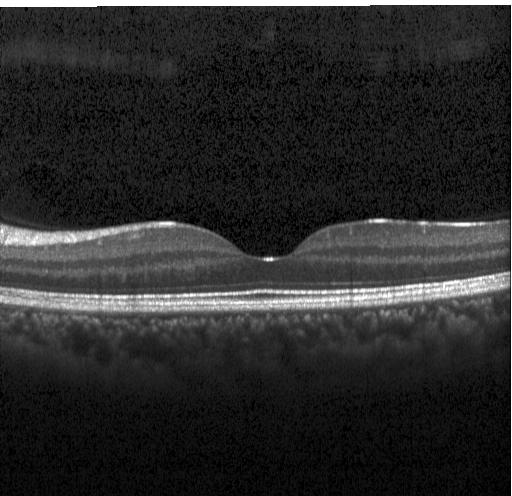
Spectral-domain optical coherence tomography; OCT B-scan; Heidelberg Spectralis. Finding: no choroidal neovascularization, no diabetic macular edema, and no drusen.